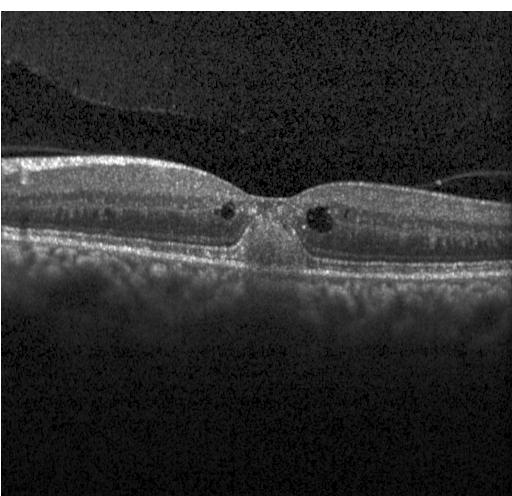

Spectral-domain OCT; centered on the fovea; retinal OCT B-scan
Impression: a choroidal neovascular membrane.